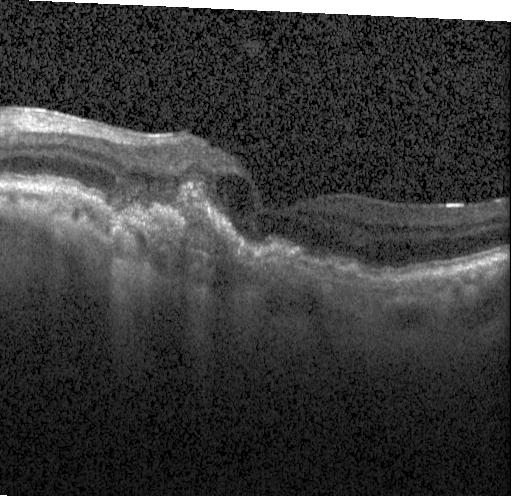
Diagnosis: choroidal neovascularization.